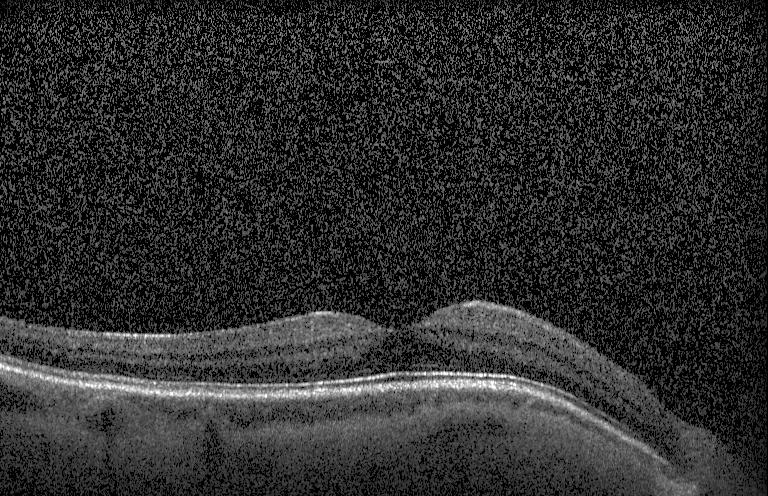 Impression: no evidence of CNV, DME, or drusen.